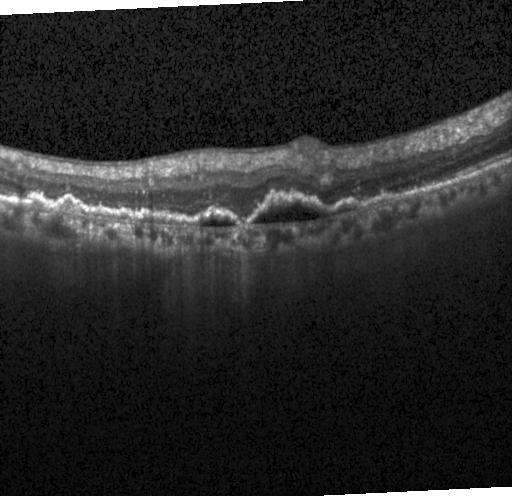 OCT line scan.
Diagnosis: a choroidal neovascular membrane.